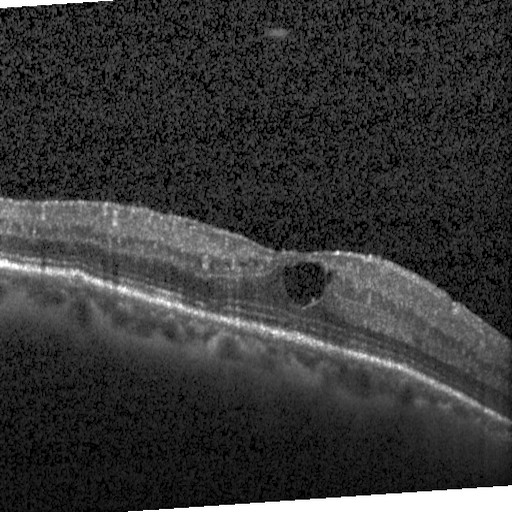
This B-scan demonstrates diabetic macular edema.